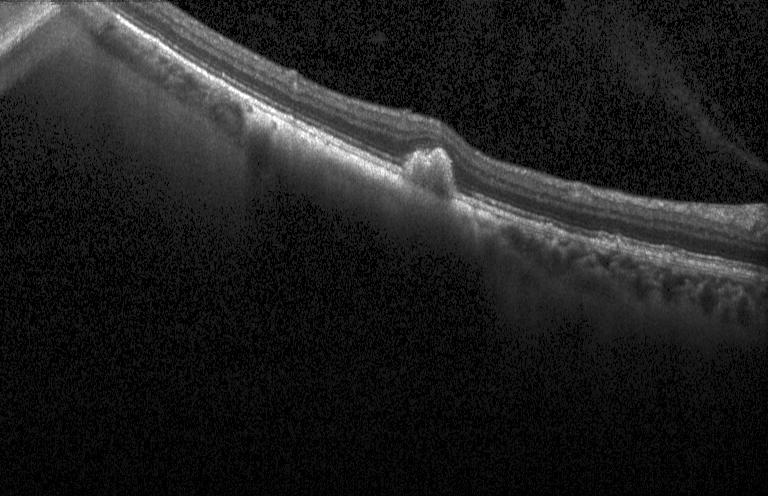 OCT finding: a choroidal neovascular membrane.